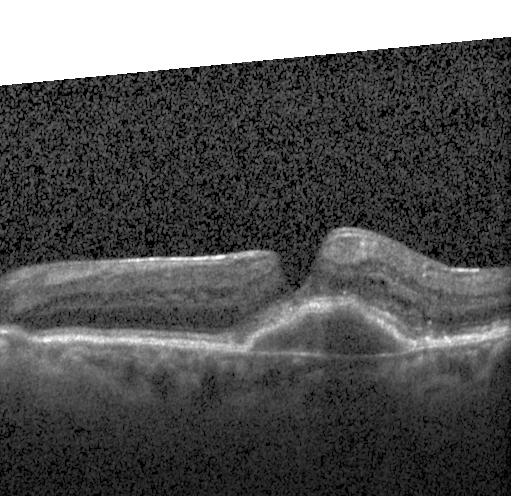
Macular OCT demonstrating a choroidal neovascular membrane.